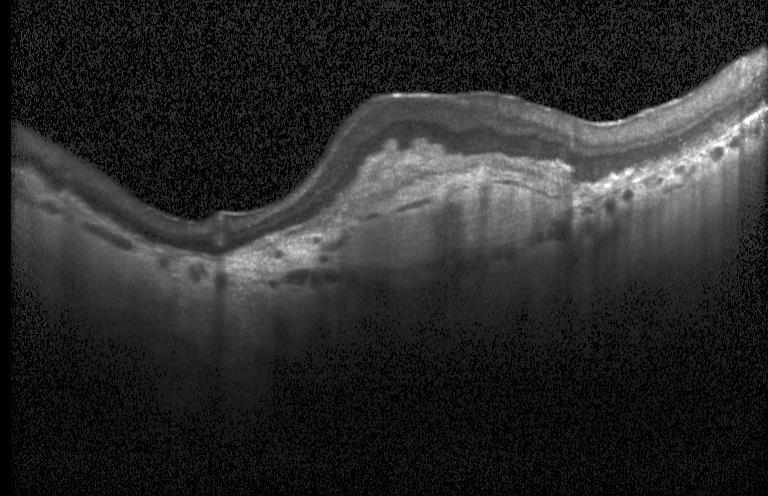 SD-OCT, macular scan, OCT line scan, instrument: Heidelberg Spectralis.
Assessment: choroidal neovascularization (CNV).